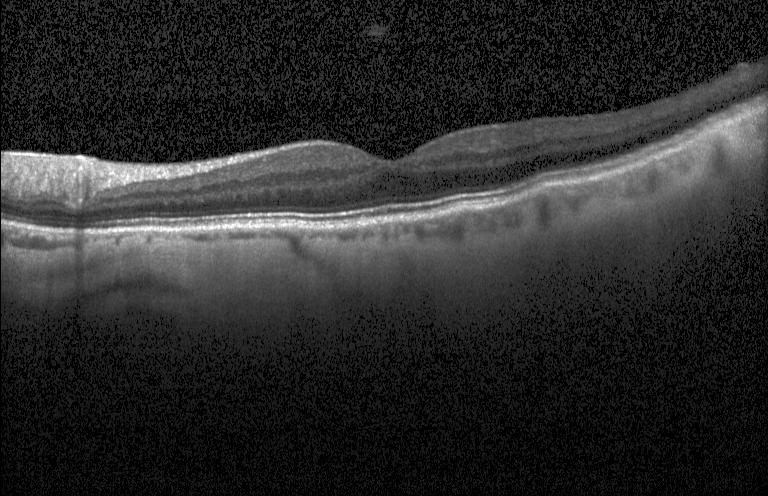
SD-OCT, retinal OCT cross-section, through the macula
Diagnosis: no CNV, no DME, and no drusen.